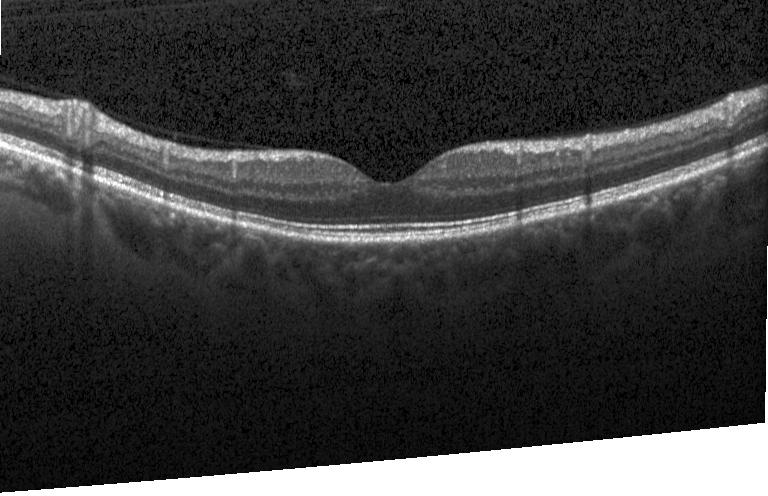

Macular OCT demonstrating no choroidal neovascularization, diabetic macular edema, or drusen.